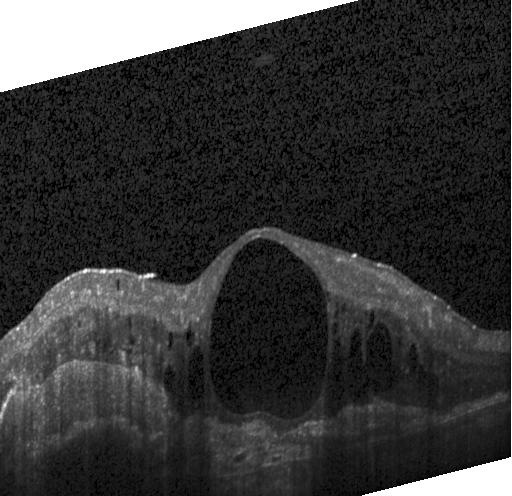

Spectral-domain OCT B-scan: a choroidal neovascular membrane.